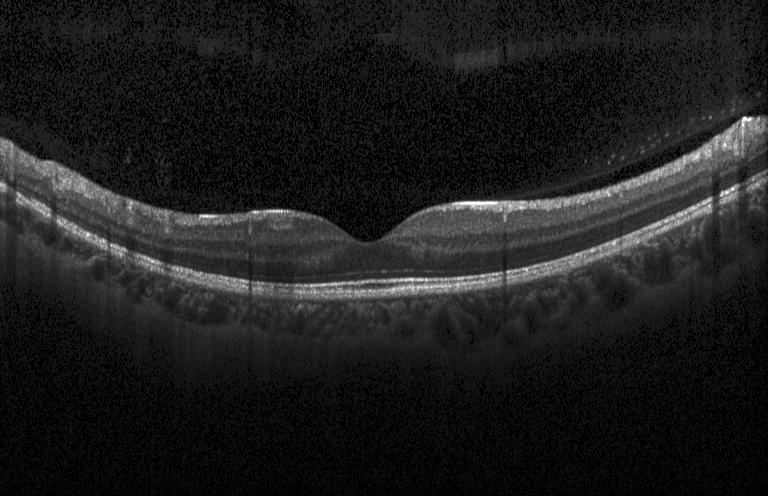 Instrument: Heidelberg Spectralis. Through the macula. Spectral-domain OCT. Retinal OCT cross-section.
Dx: neither choroidal neovascularization, diabetic macular edema, nor drusen.